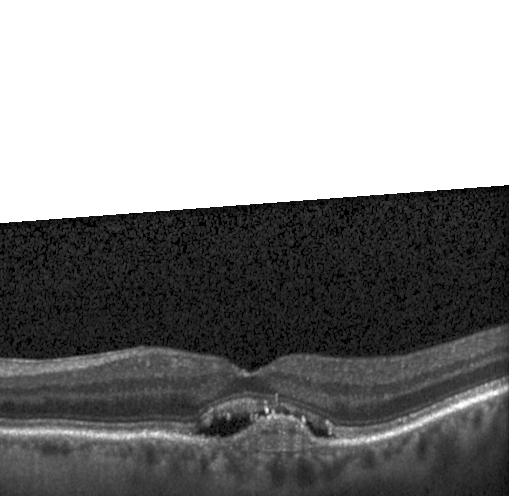
Finding: a choroidal neovascular membrane.